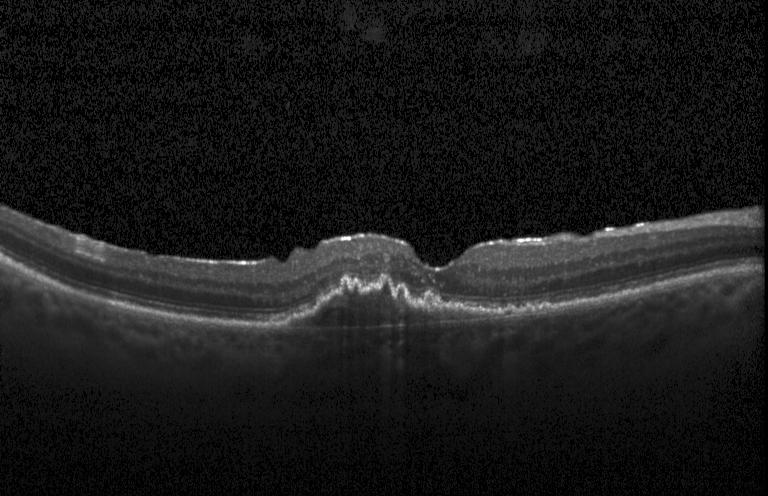 Spectral-domain OCT B-scan: a choroidal neovascular membrane.